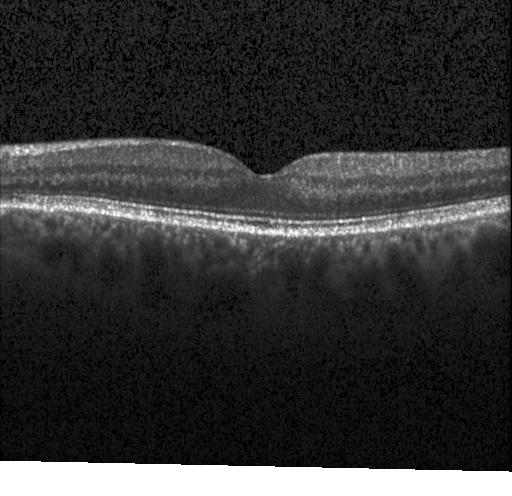 Optical coherence tomography scan. Impression: neither choroidal neovascularization, diabetic macular edema, nor drusen.